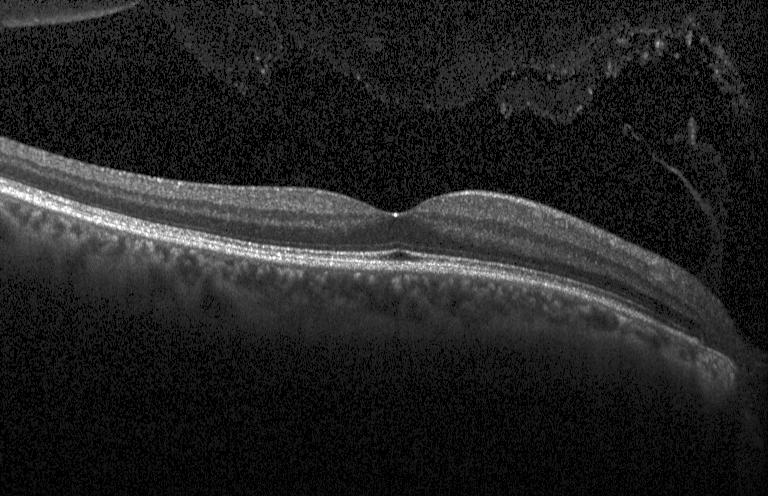
Retinal OCT B-scan. Heidelberg Spectralis
No choroidal neovascularization, diabetic macular edema, or drusen.